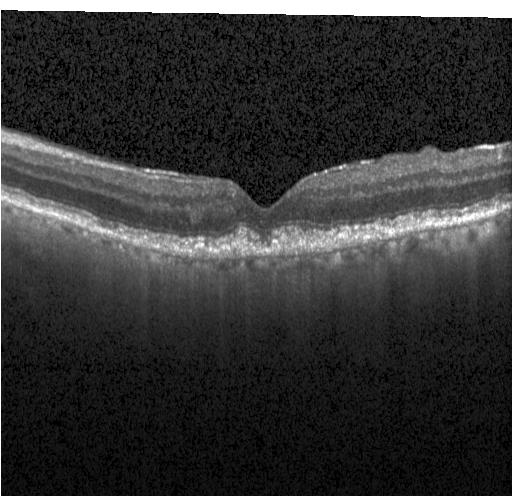 Finding: multiple drusen.